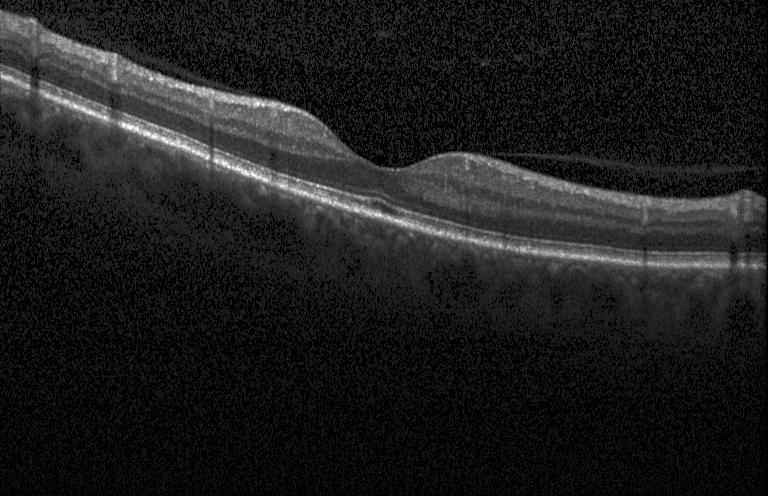

Heidelberg Spectralis · macular scan · SD-OCT · retinal OCT B-scan. Neither CNV, DME, nor drusen.